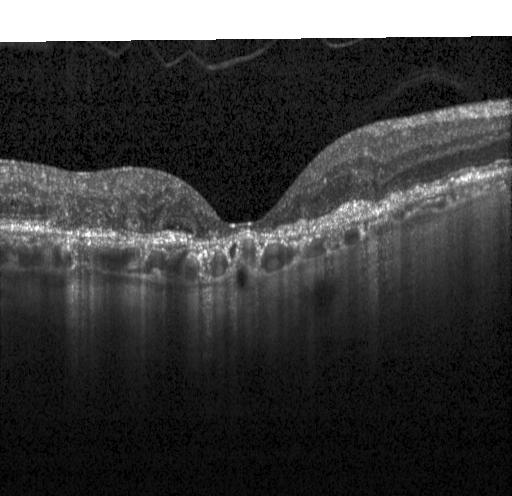

The scan shows a choroidal neovascular membrane.